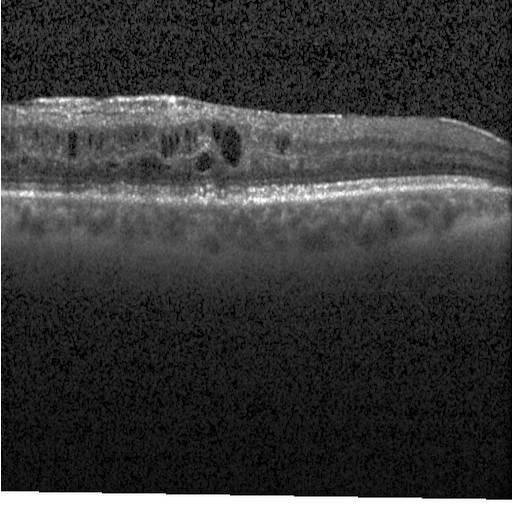
Spectral-domain optical coherence tomography, Heidelberg Spectralis OCT system, horizontal scan through the fovea, retinal OCT cross-section.
DME.